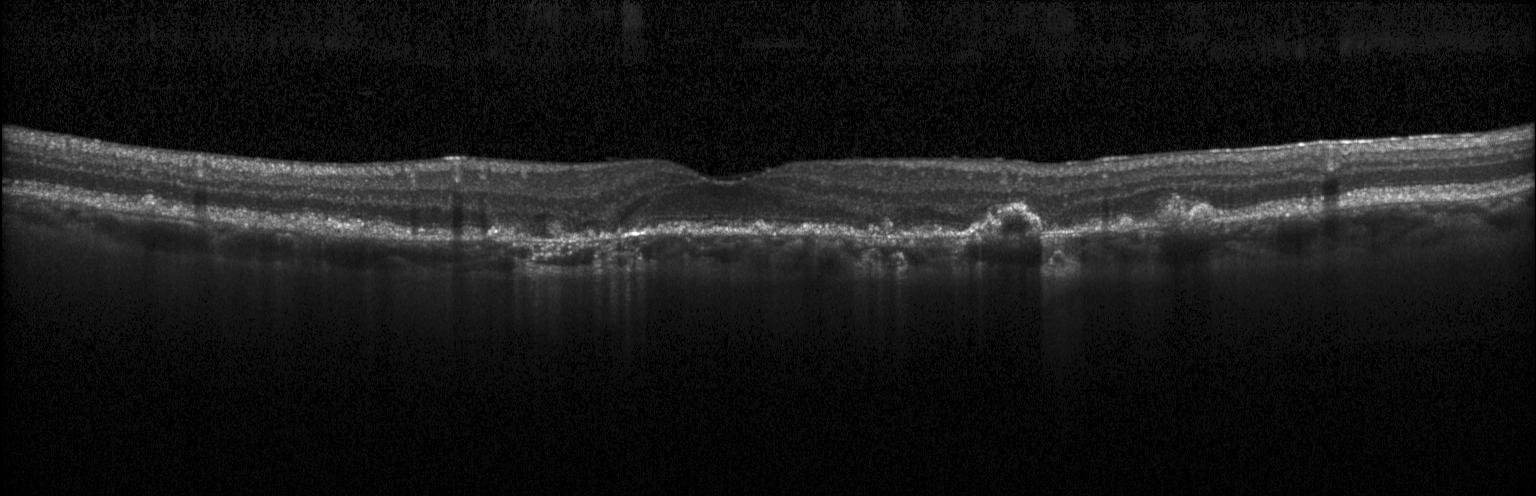

Impression: a choroidal neovascular membrane.